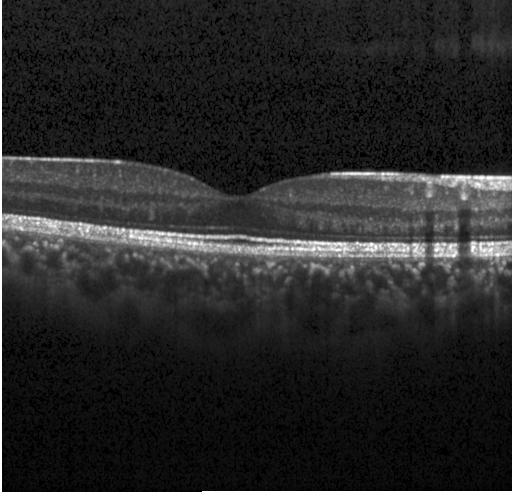 Retinal OCT cross-section showing no CNV, no DME, and no drusen.